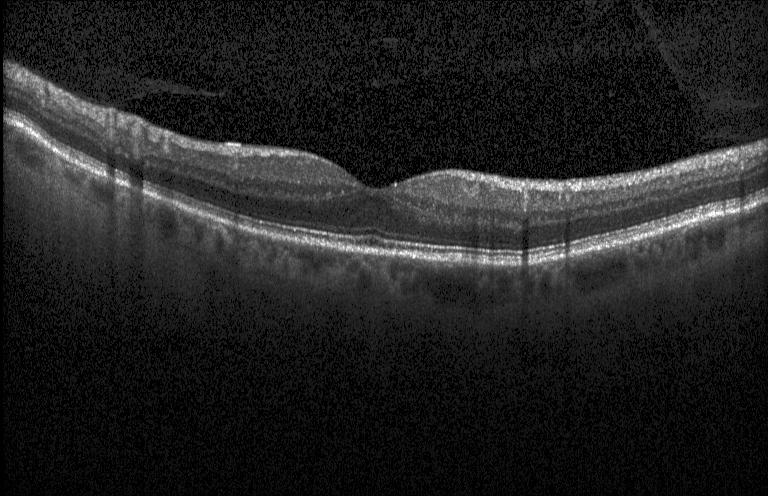
Macular OCT: neither choroidal neovascularization, diabetic macular edema, nor drusen.